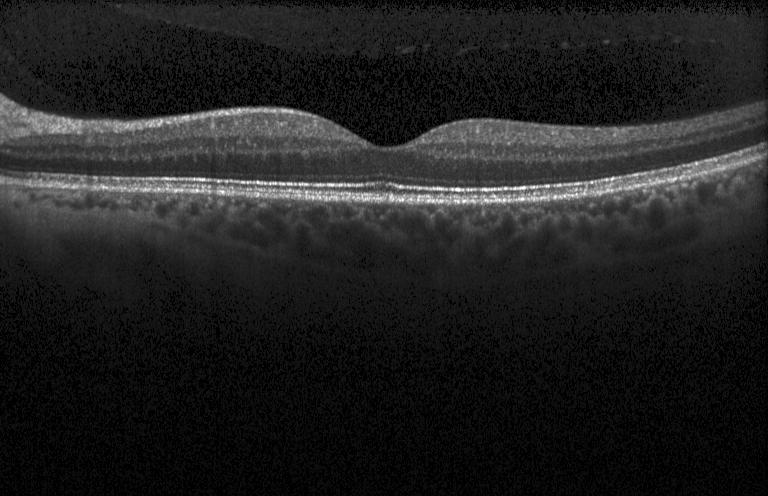

Assessment: no choroidal neovascularization, diabetic macular edema, or drusen.